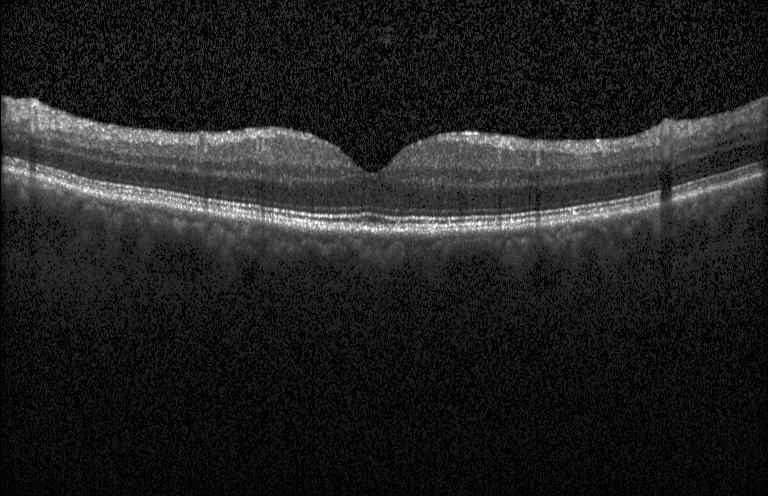
Through the macula; OCT line scan; Heidelberg Spectralis; SD-OCT
Finding: no CNV, DME, or drusen.